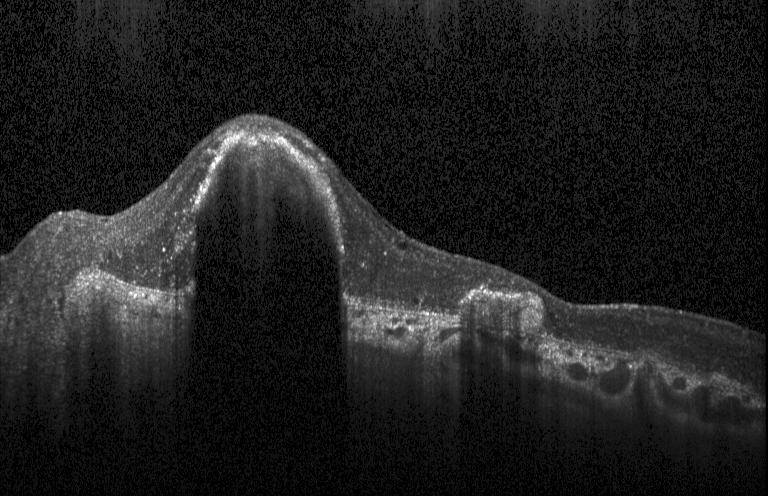

Impression: a choroidal neovascular membrane.